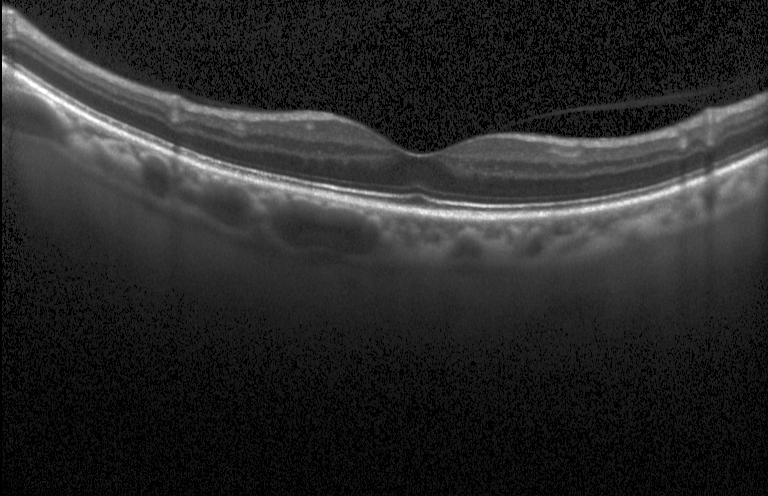 Fovea-centered · optical coherence tomography B-scan · instrument: Heidelberg Spectralis — The scan shows no evidence of choroidal neovascularization, diabetic macular edema, or drusen.